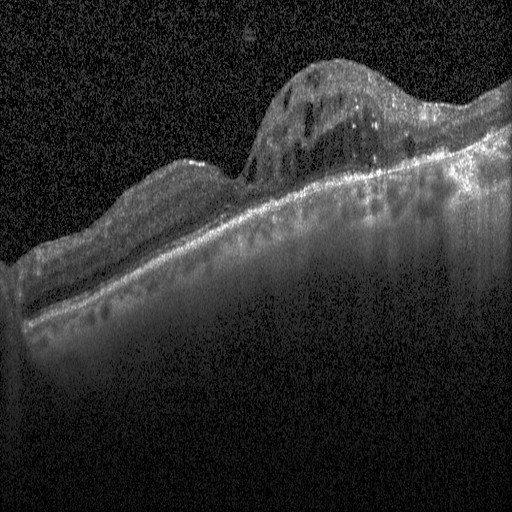
Optical coherence tomography B-scan
Diagnosis: DME.